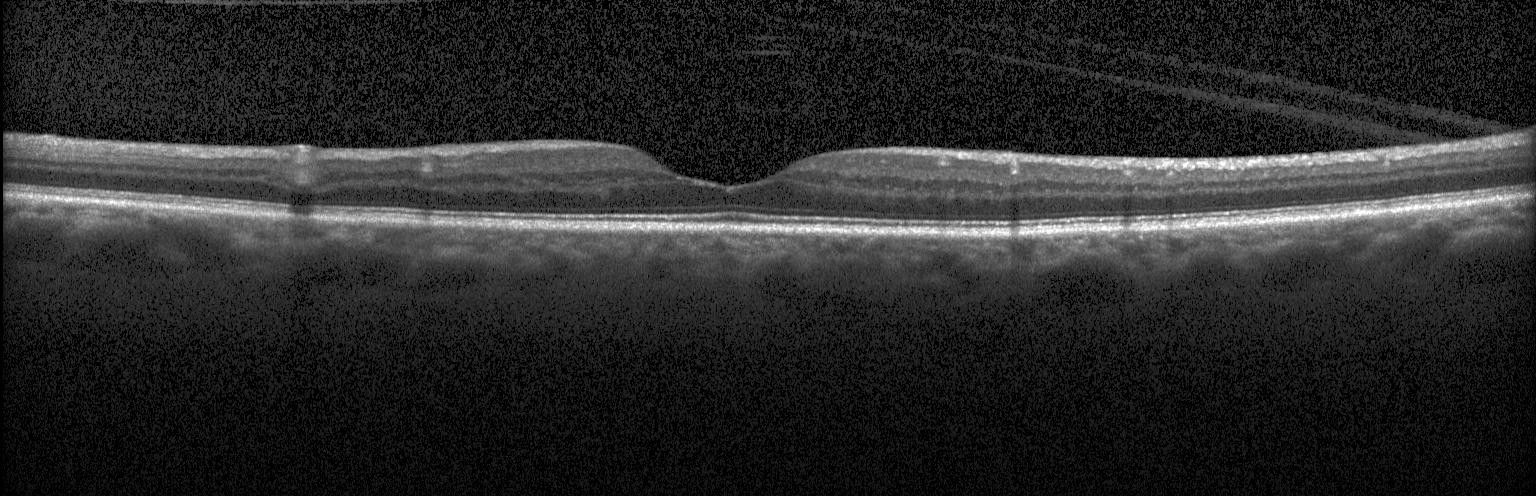

No CNV, DME, or drusen.